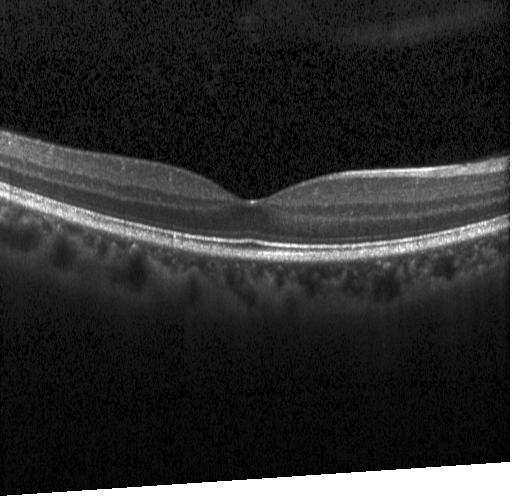

Through the macula; OCT line scan; spectral-domain OCT
Impression: no CNV, no DME, and no drusen.